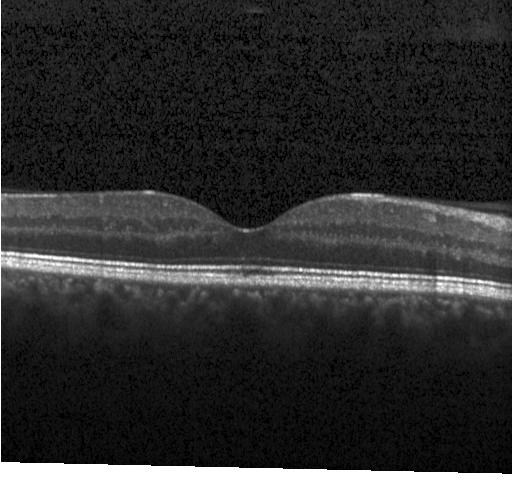

Fovea-centered · OCT line scan · Heidelberg Spectralis OCT system.
Finding: no choroidal neovascularization, no diabetic macular edema, and no drusen.